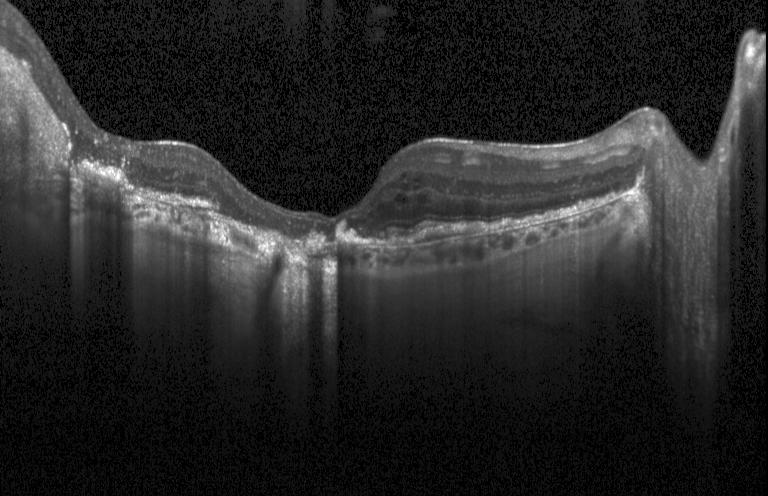

Optical coherence tomography scan — Diagnosis: CNV.